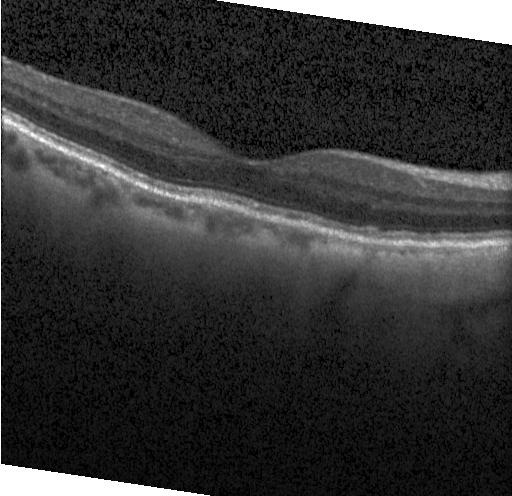
Instrument: Heidelberg Spectralis. OCT line scan. Centered on the fovea — Diagnosis: neither choroidal neovascularization, diabetic macular edema, nor drusen.